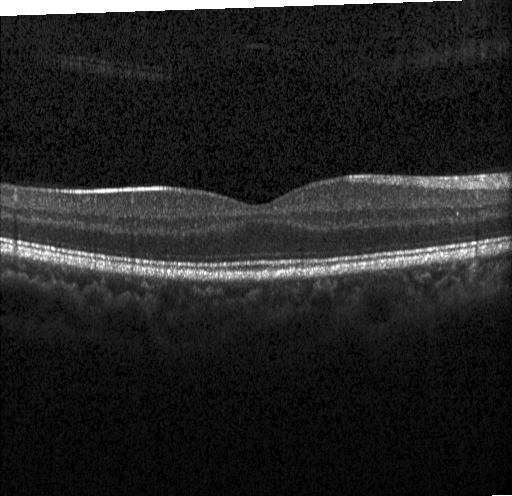
Optical coherence tomography scan, acquired on a Heidelberg Spectralis, SD-OCT
No evidence of choroidal neovascularization, diabetic macular edema, or drusen.